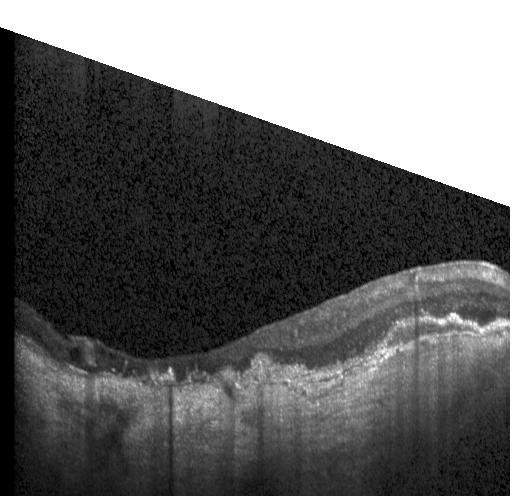 Dx: a choroidal neovascular membrane.